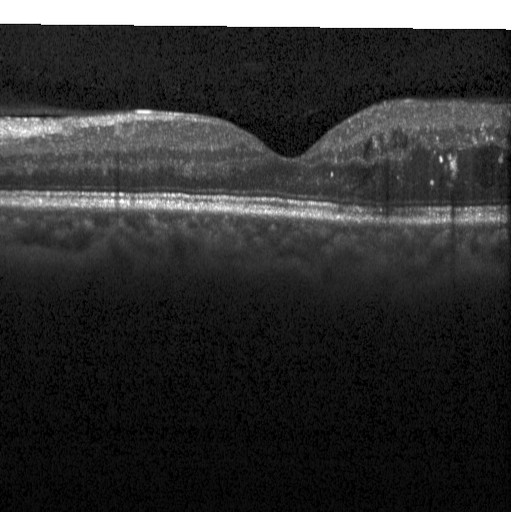
OCT B-scan showing diabetic macular edema (DME).